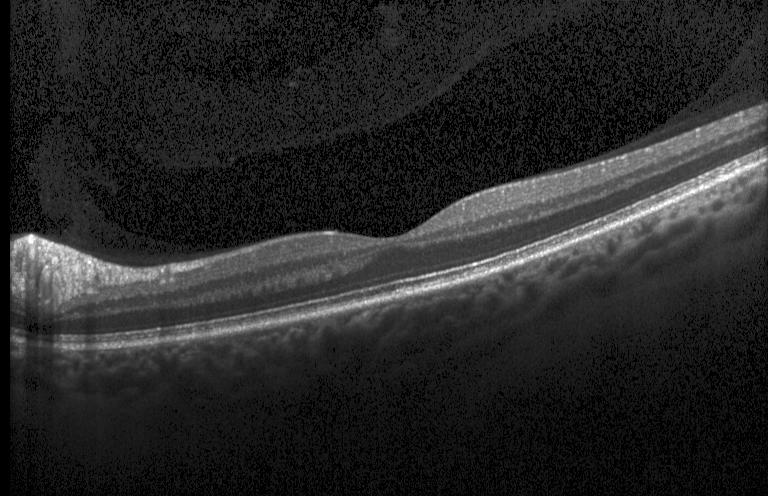 Retinal OCT cross-section showing neither choroidal neovascularization, diabetic macular edema, nor drusen.